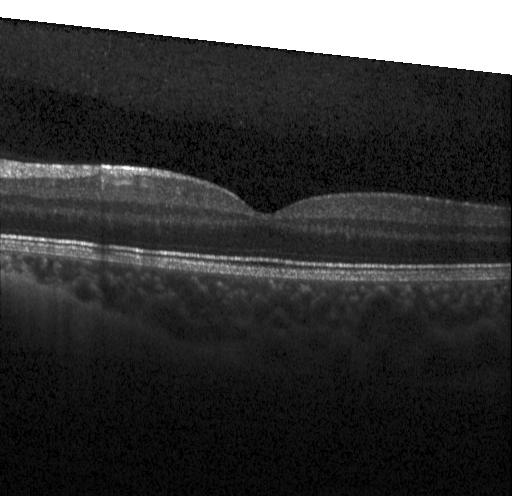

Optical coherence tomography scan.
The scan shows no choroidal neovascularization, diabetic macular edema, or drusen.